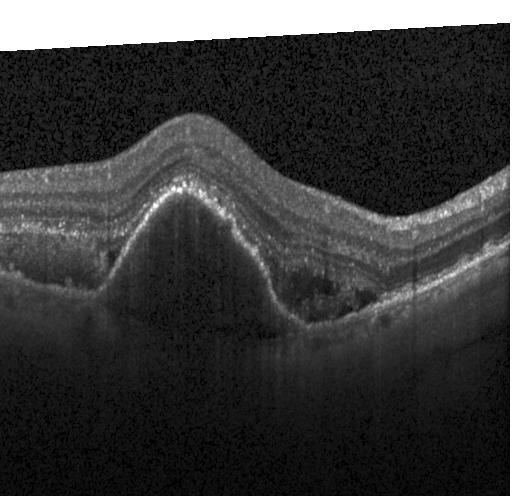
Diagnosis: choroidal neovascularization.